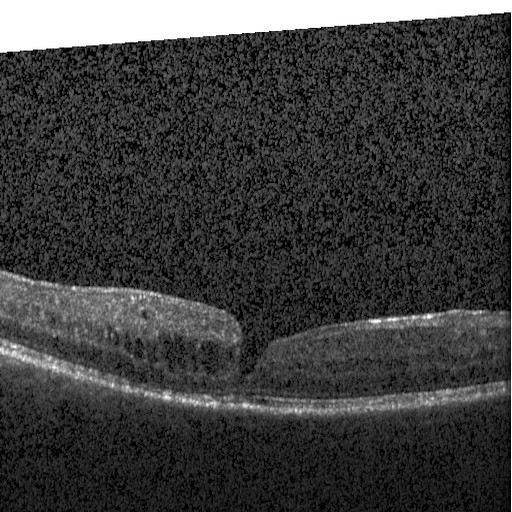

Retinal OCT cross-section showing diabetic macular edema (DME).